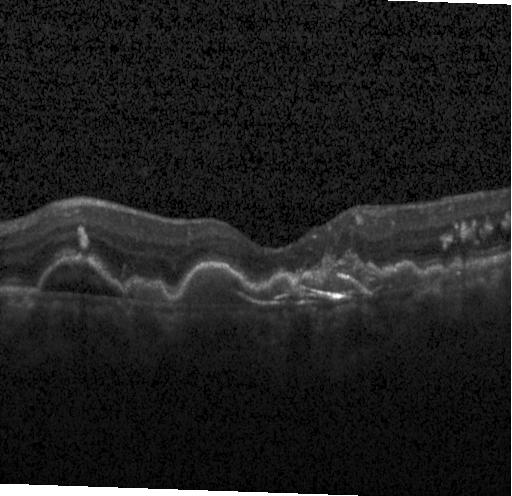
Diagnosis: CNV.